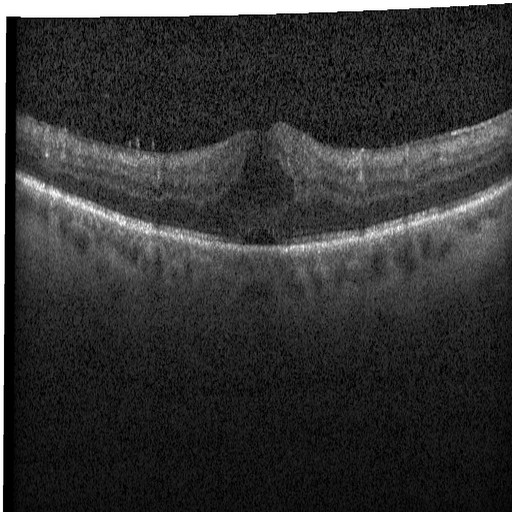

Spectral-domain optical coherence tomography. Optical coherence tomography B-scan. Horizontal scan through the fovea. Heidelberg Spectralis. Impression: diabetic macular edema.